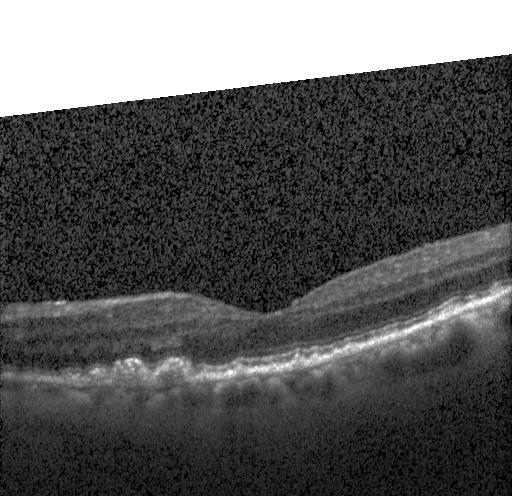 Multiple drusen.